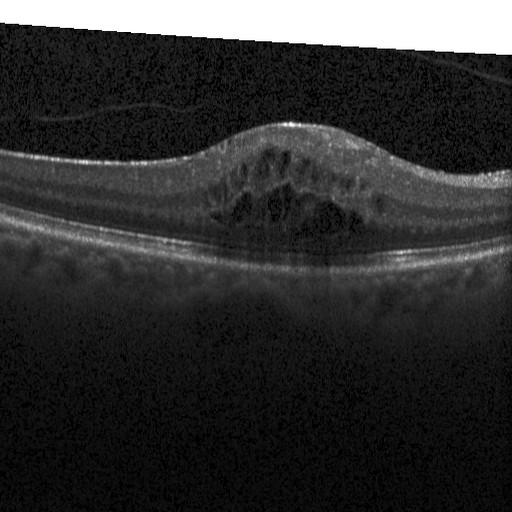 Dx: diabetic macular edema.